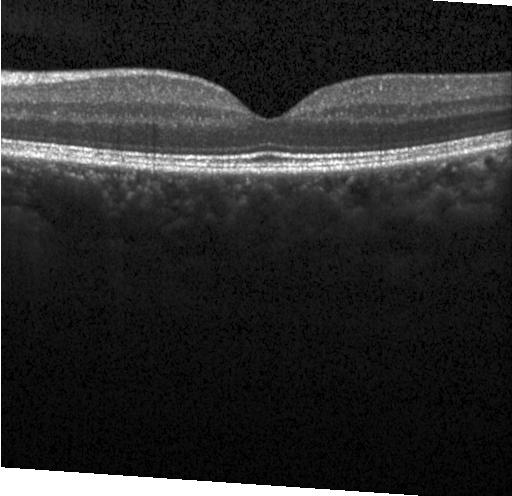 Finding: no choroidal neovascularization, no diabetic macular edema, and no drusen.